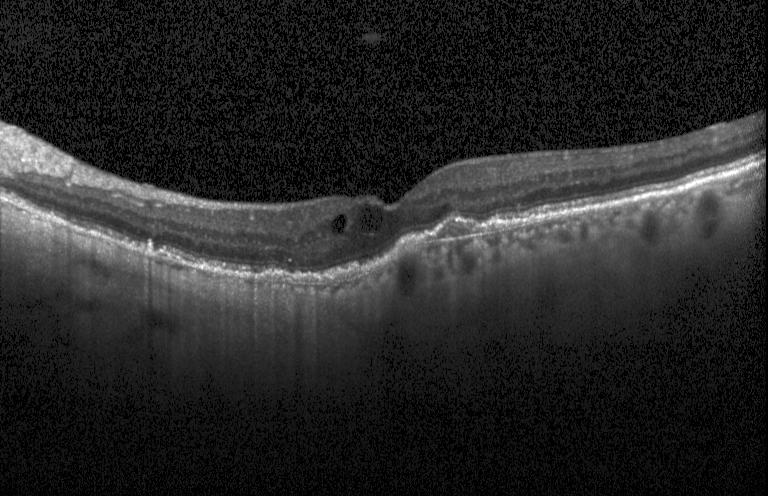

This B-scan demonstrates a choroidal neovascular membrane.